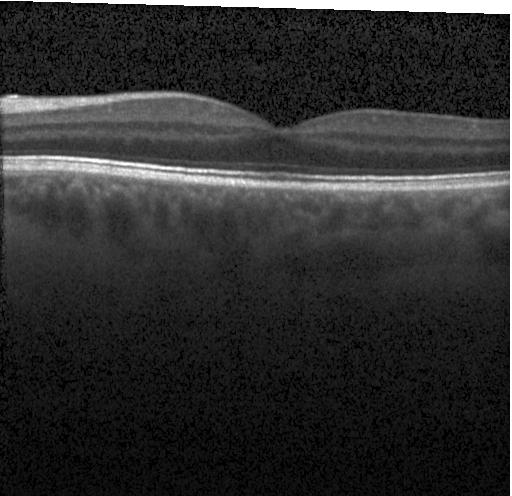 Assessment: no CNV, DME, or drusen.